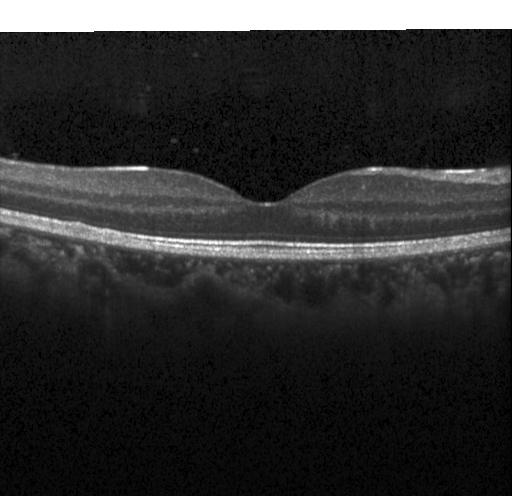
Heidelberg Spectralis OCT system. Spectral-domain optical coherence tomography. Optical coherence tomography scan. Macular scan. Dx: neither CNV, DME, nor drusen.